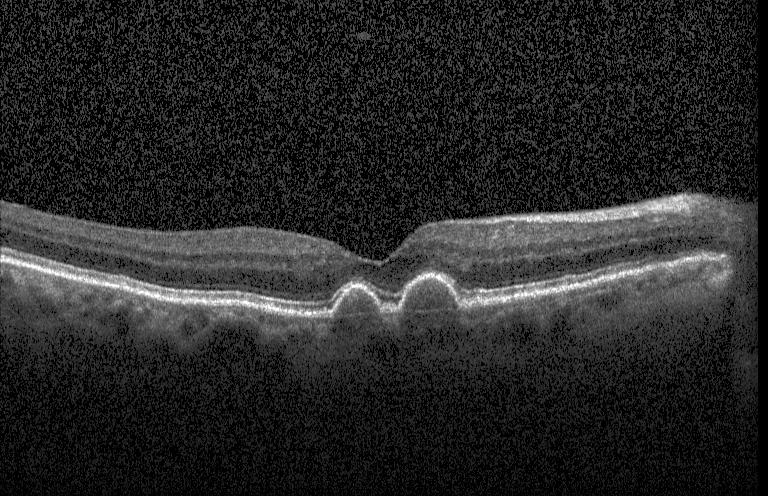
OCT B-scan · spectral-domain OCT — Finding: drusen.